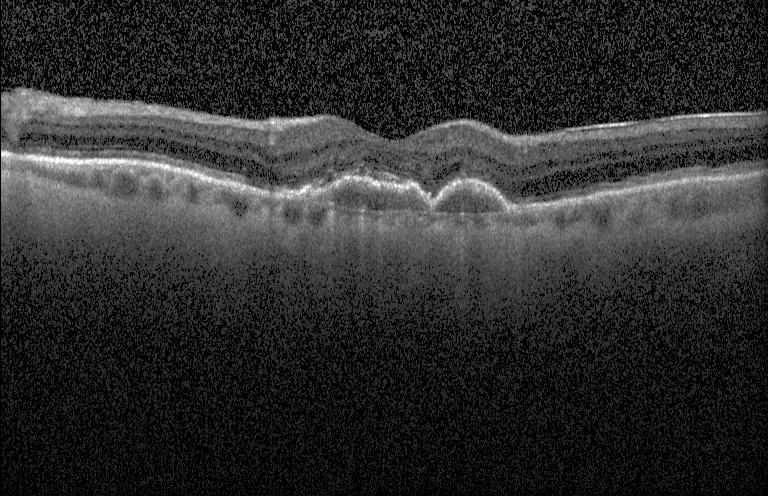 Heidelberg Spectralis; spectral-domain OCT; through the macula; retinal OCT cross-section
Impression: choroidal neovascularization (CNV).